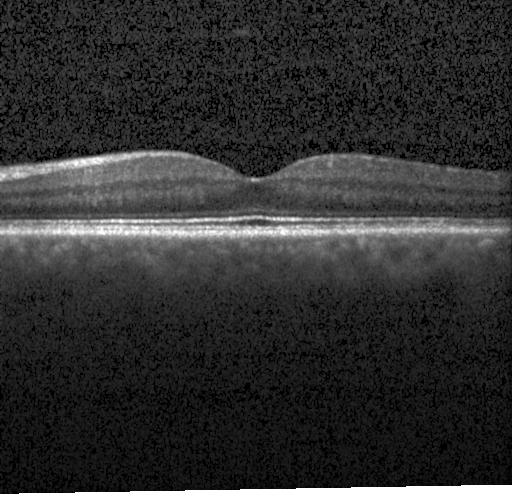

Retinal OCT cross-section showing no choroidal neovascularization, diabetic macular edema, or drusen.